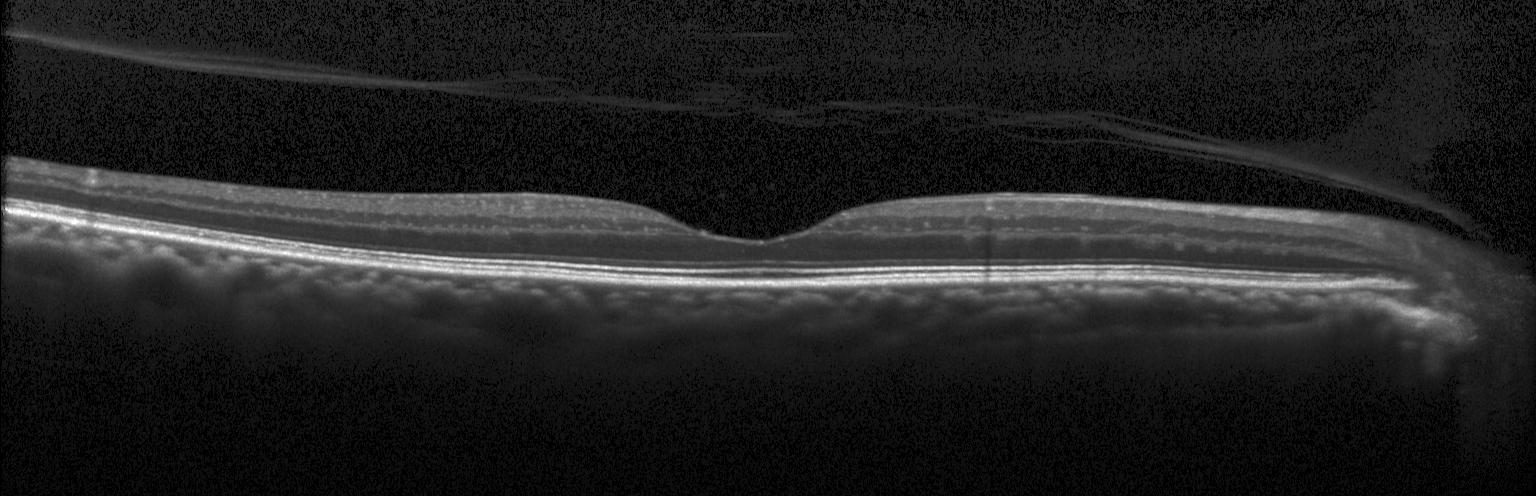 SD-OCT, retinal OCT cross-section, acquired on a Heidelberg Spectralis. The scan shows no CNV, DME, or drusen.